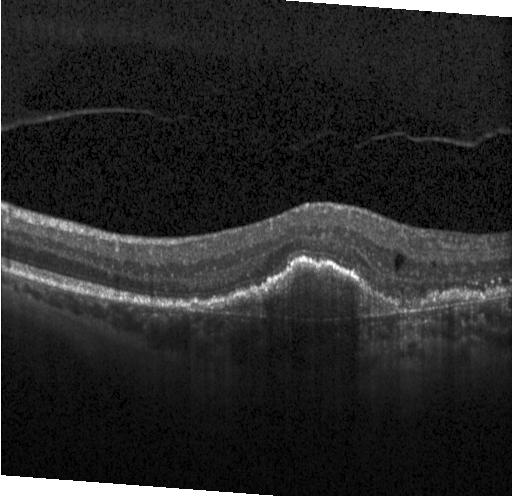 OCT B-scan. Macular OCT: CNV.